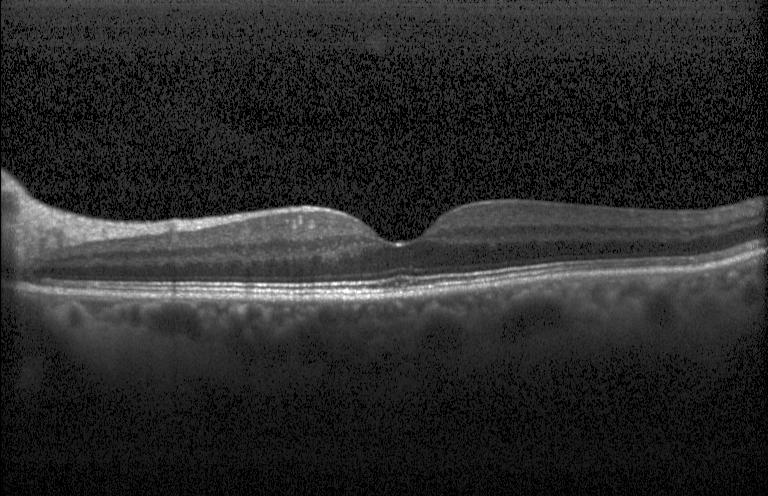

Finding: no evidence of choroidal neovascularization, diabetic macular edema, or drusen.